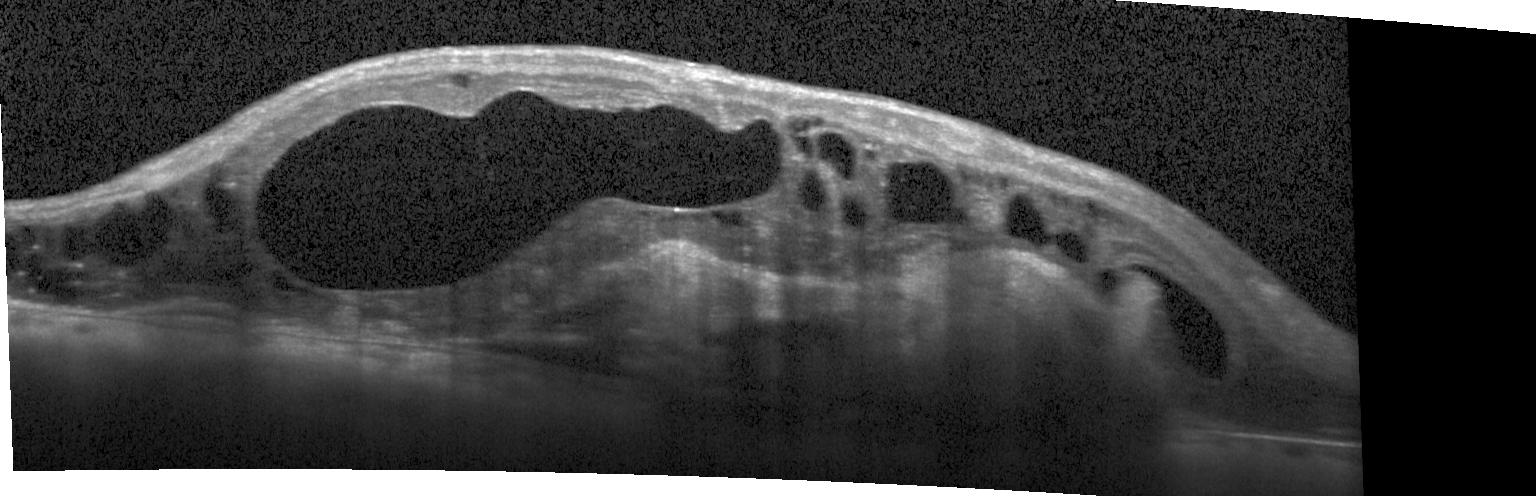 Through the macula, retinal OCT B-scan — Finding: CNV.